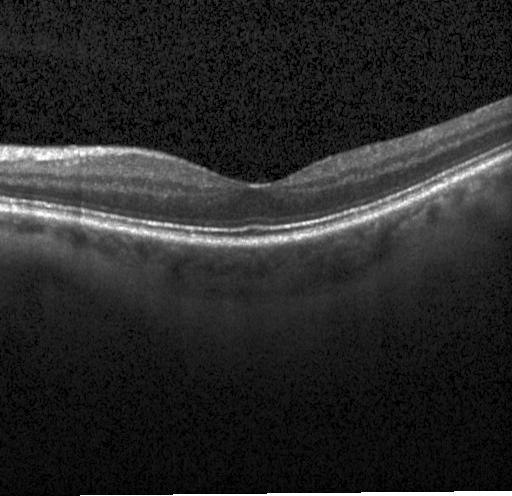
Horizontal scan through the fovea; retinal OCT B-scan — This B-scan demonstrates neither CNV, DME, nor drusen.